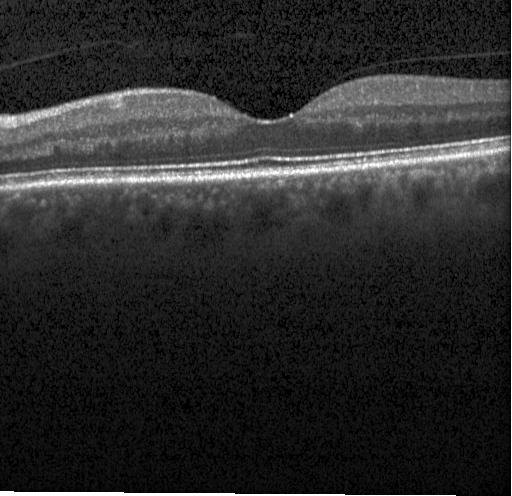 OCT line scan. Acquired on a Heidelberg Spectralis — Finding: no choroidal neovascularization, no diabetic macular edema, and no drusen.